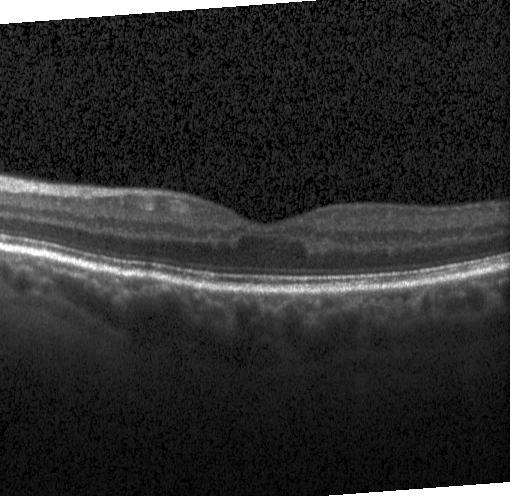

Spectral-domain OCT B-scan: no choroidal neovascularization, diabetic macular edema, or drusen.